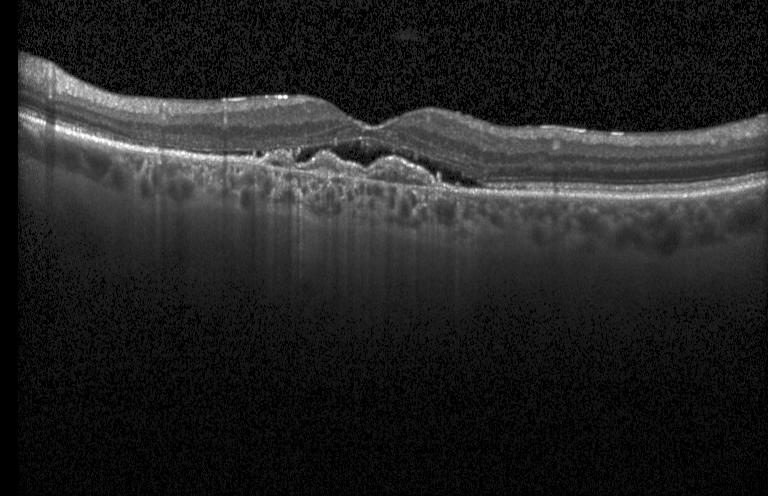 Macular OCT: choroidal neovascularization (CNV).